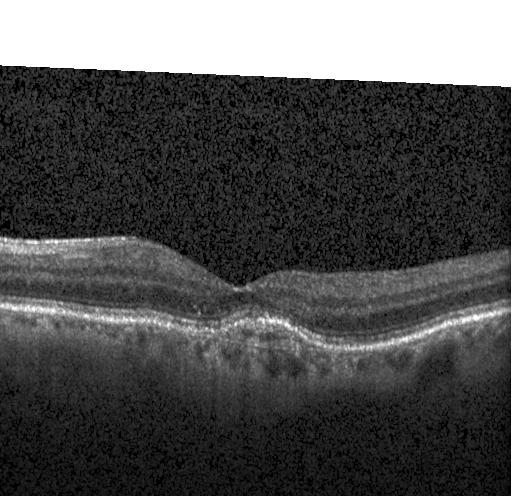

Heidelberg Spectralis, optical coherence tomography scan, fovea-centered, spectral-domain OCT — Diagnosis: a choroidal neovascular membrane.